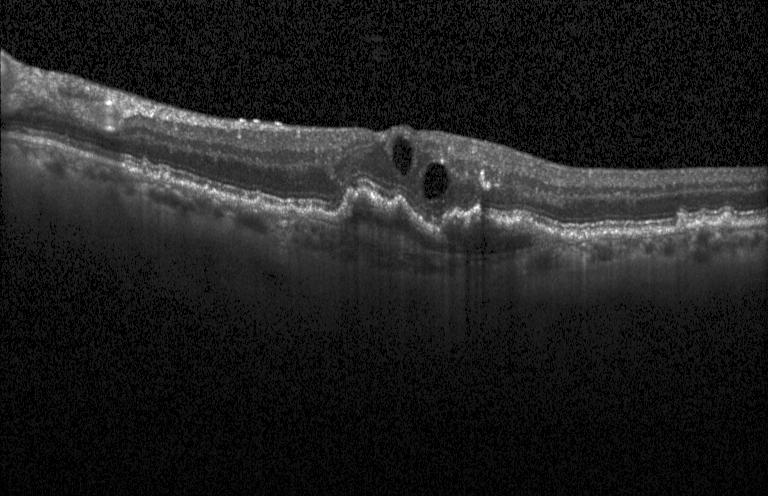
Macular OCT demonstrating choroidal neovascularization.